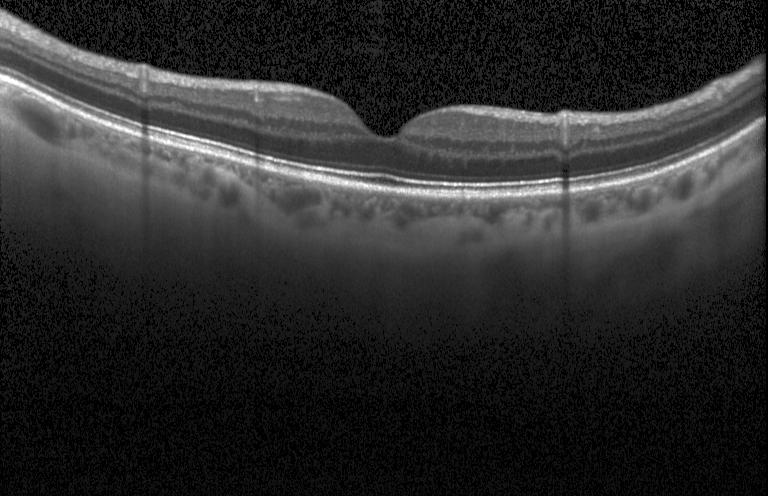

Retinal OCT B-scan; fovea-centered. Diagnosis: no evidence of choroidal neovascularization, diabetic macular edema, or drusen.